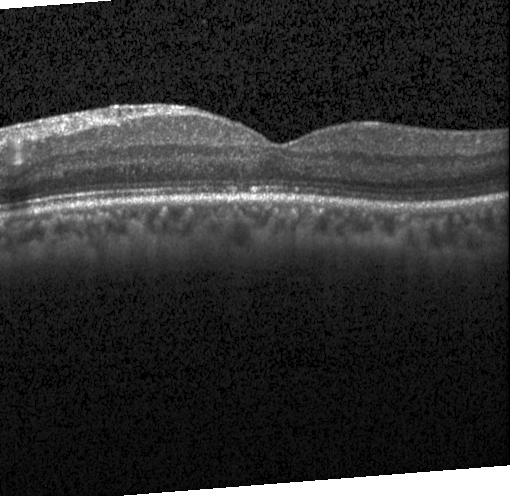

SD-OCT. Heidelberg Spectralis. Optical coherence tomography scan.
Impression: no CNV, no DME, and no drusen.